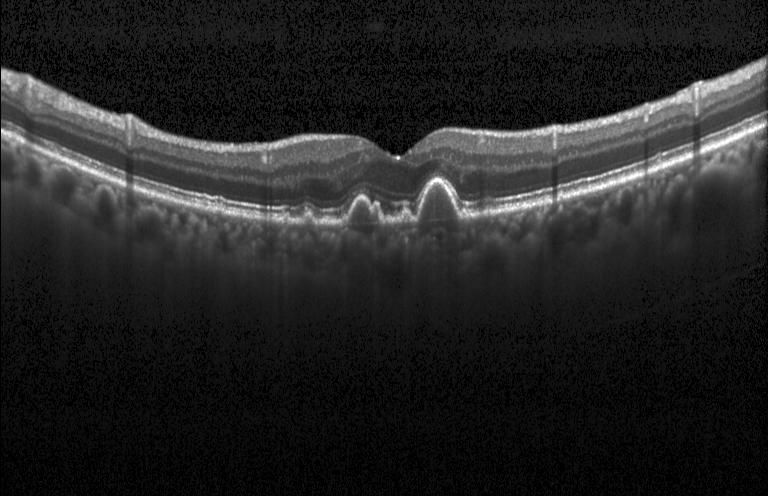

OCT B-scan, through the macula, Heidelberg Spectralis.
The scan shows drusen.